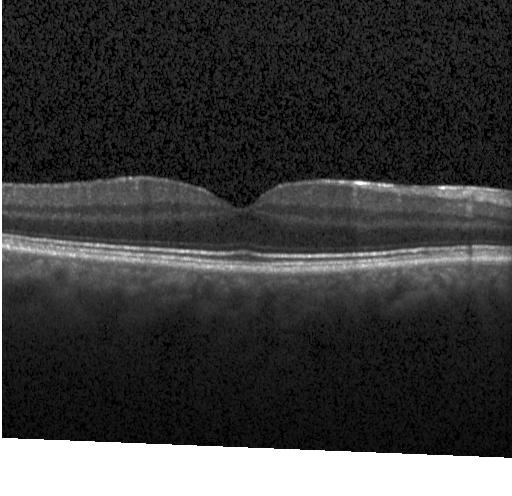

OCT line scan. This B-scan demonstrates no choroidal neovascularization, diabetic macular edema, or drusen.